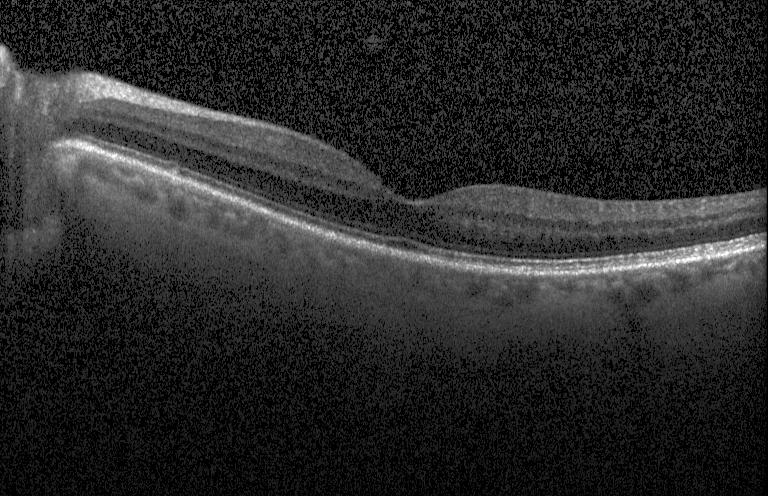
Macular scan; retinal OCT cross-section; Heidelberg Spectralis; spectral-domain OCT. Impression: no choroidal neovascularization, no diabetic macular edema, and no drusen.